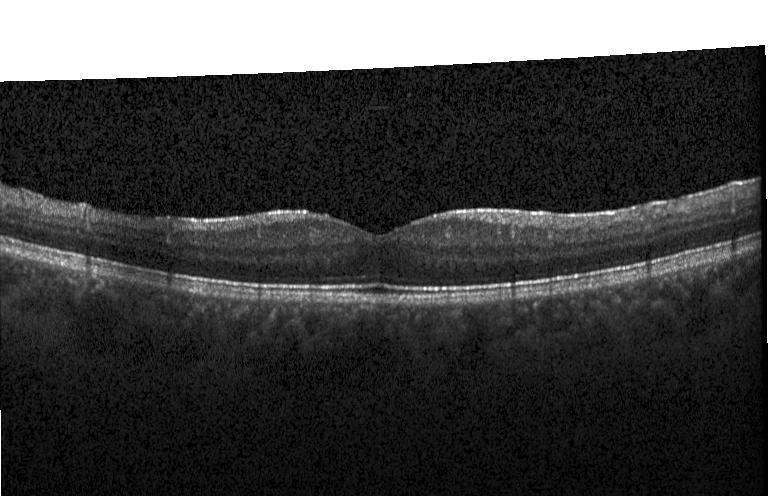 Optical coherence tomography scan. Macular OCT: neither choroidal neovascularization, diabetic macular edema, nor drusen.